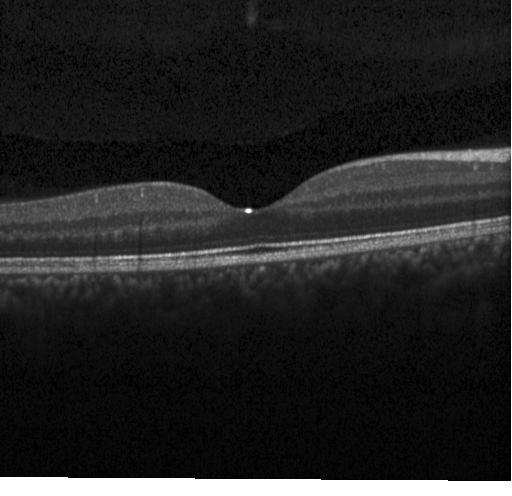 Heidelberg Spectralis OCT system, retinal OCT B-scan, through the macula, spectral-domain OCT. Diagnosis: no choroidal neovascularization, no diabetic macular edema, and no drusen.